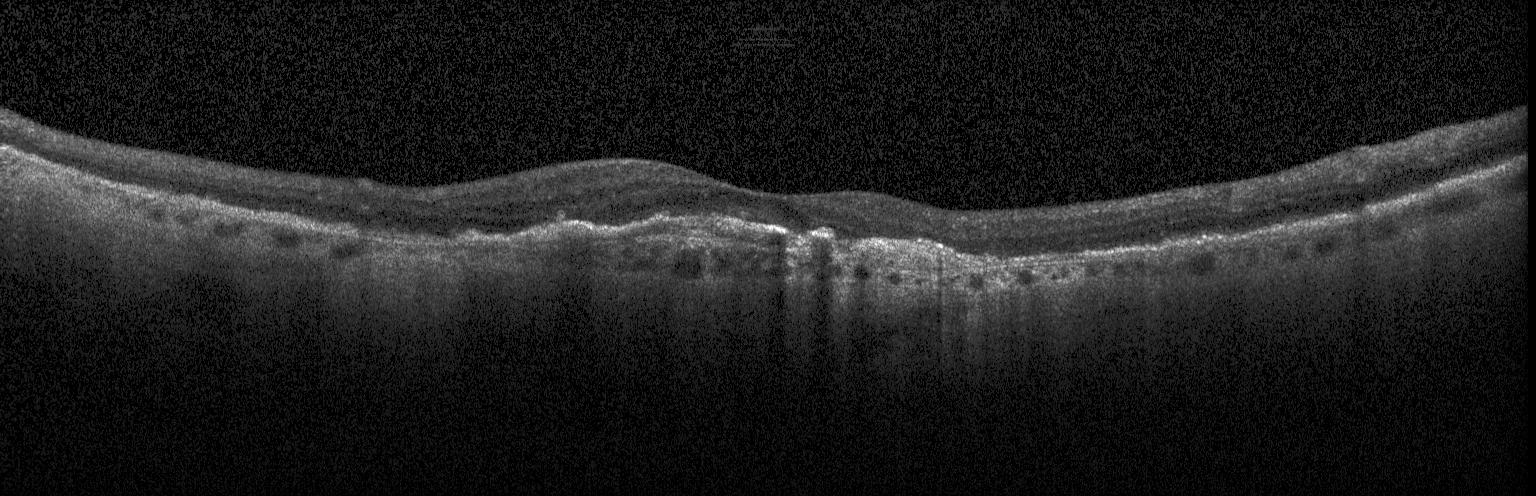 Retinal OCT B-scan — This B-scan demonstrates choroidal neovascularization.